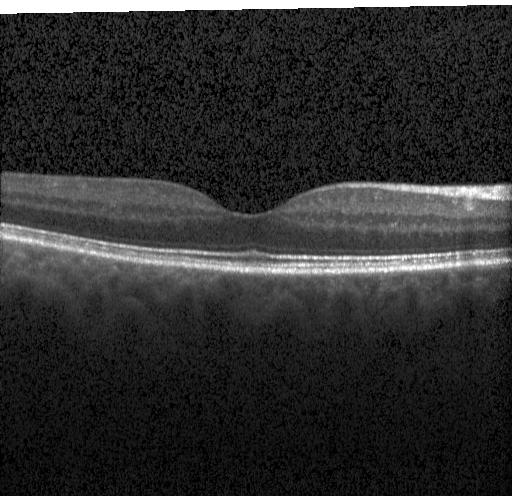

Impression: neither choroidal neovascularization, diabetic macular edema, nor drusen.